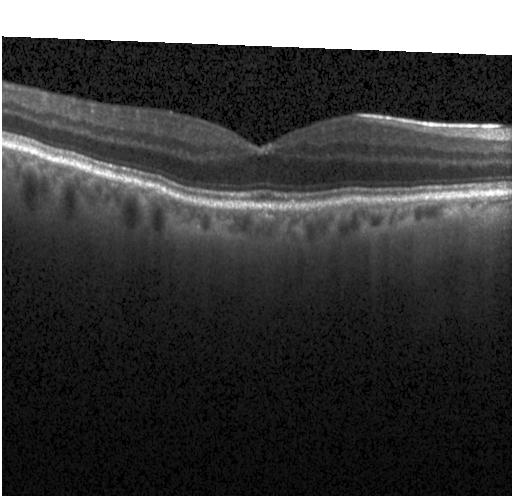 Impression: no choroidal neovascularization, no diabetic macular edema, and no drusen.